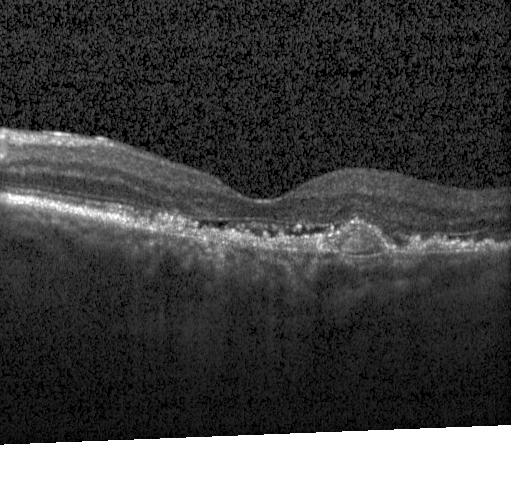

Macular OCT demonstrating a choroidal neovascular membrane.